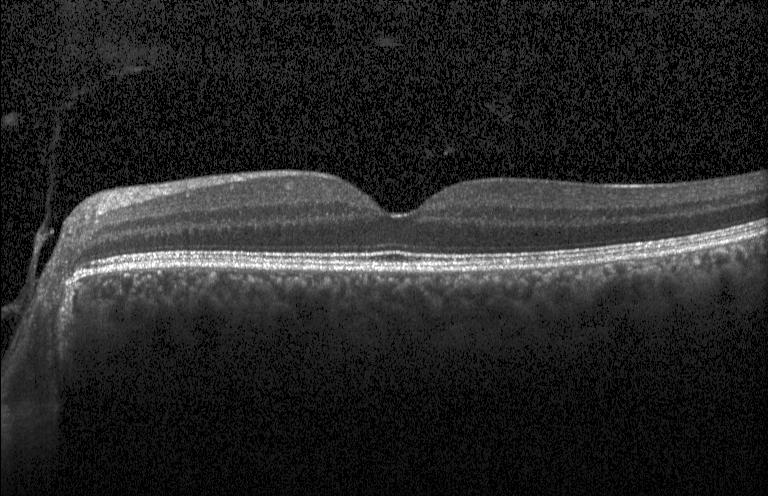

Retinal OCT cross-section · spectral-domain OCT
OCT finding: no choroidal neovascularization, no diabetic macular edema, and no drusen.